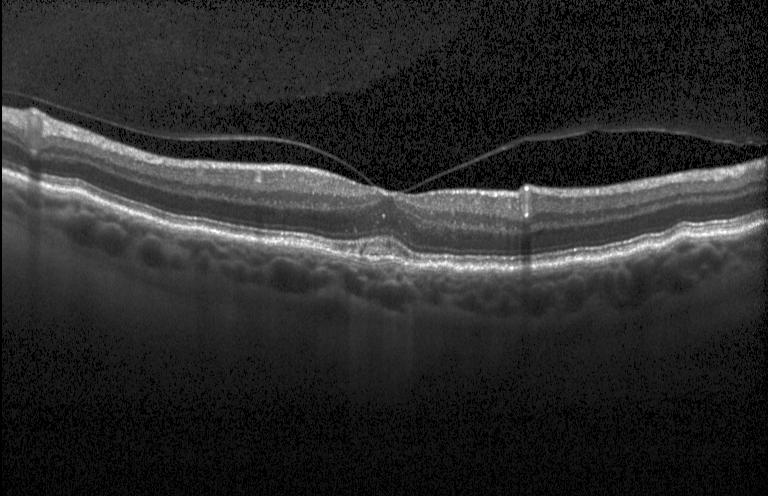

Sub-RPE drusenoid deposits.